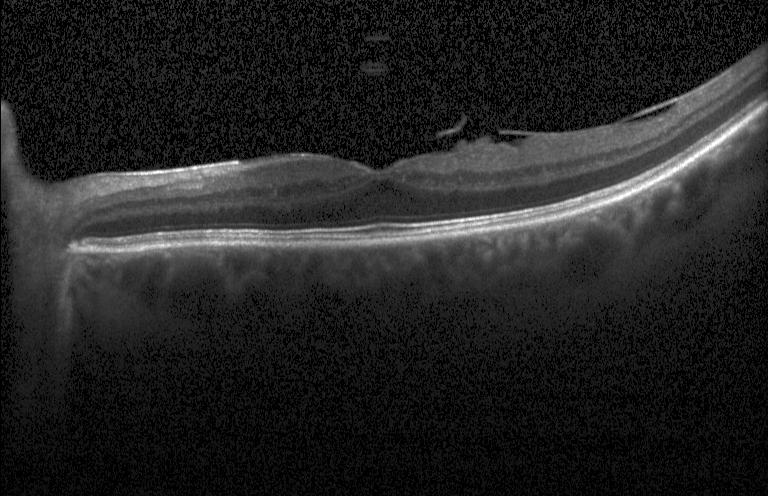

SD-OCT, acquired on a Heidelberg Spectralis, OCT line scan, through the macula
Macular OCT: no choroidal neovascularization, no diabetic macular edema, and no drusen.